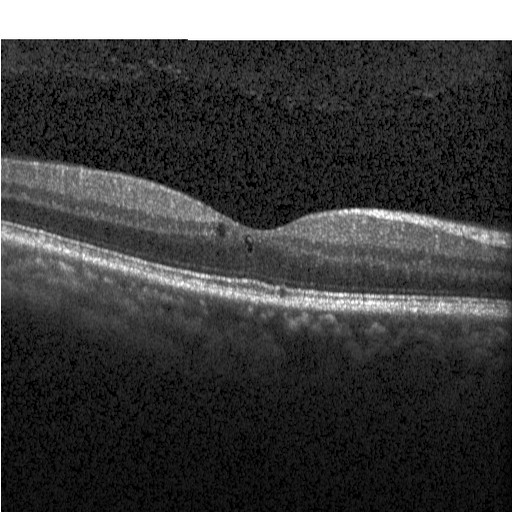

Retinal OCT cross-section.
Diagnosis: diabetic macular edema (DME).